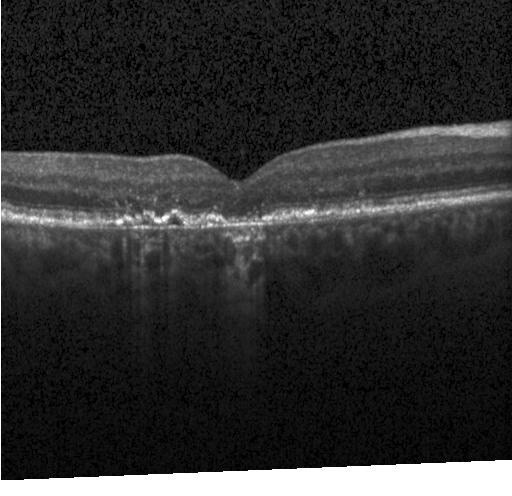 Optical coherence tomography B-scan, SD-OCT, macular scan, instrument: Heidelberg Spectralis. Finding: a choroidal neovascular membrane.